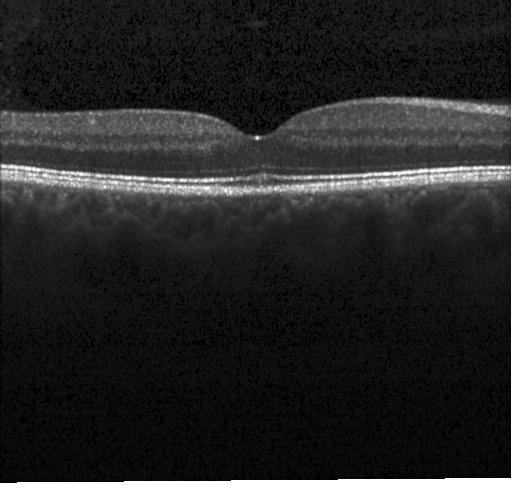

OCT scan showing no CNV, no DME, and no drusen.